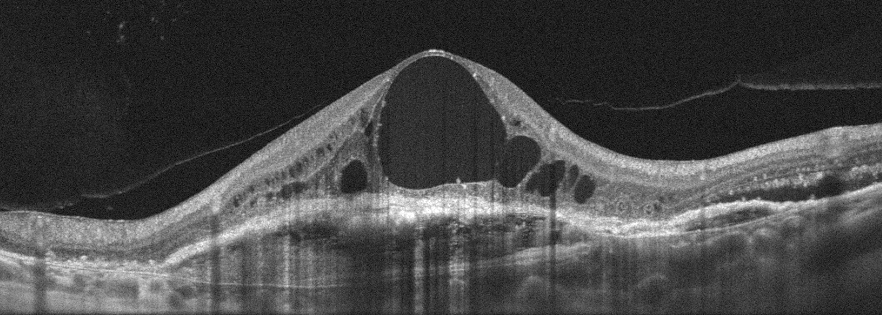
Optical coherence tomography B-scan, oculus dexter — Diagnosis: AMD.